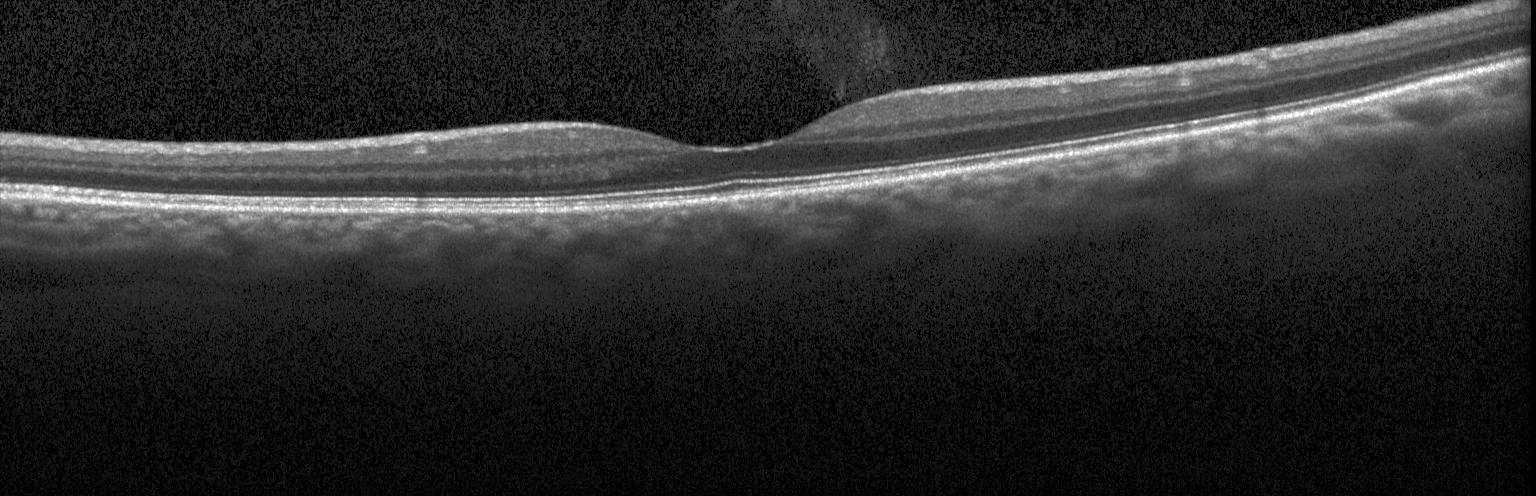

Dx: no choroidal neovascularization, diabetic macular edema, or drusen.